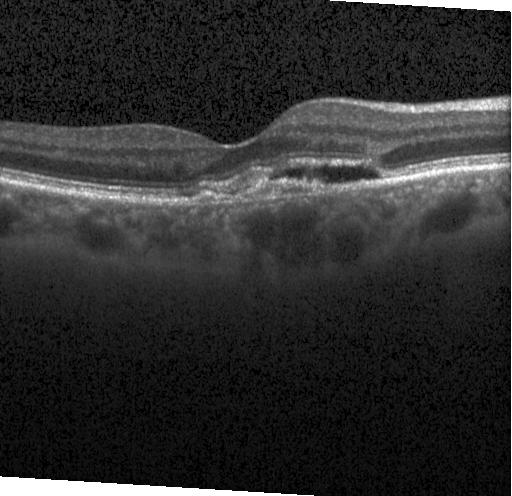 Assessment: a choroidal neovascular membrane.